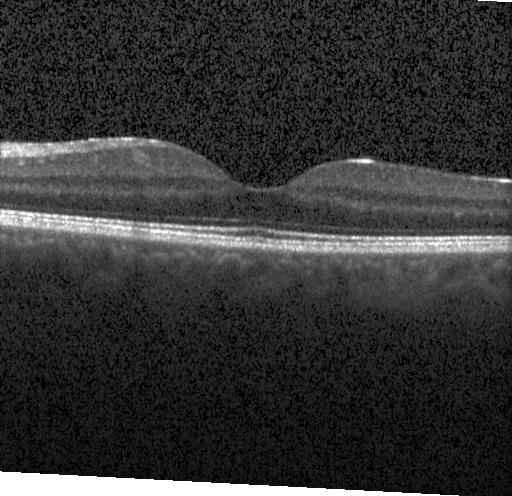

OCT scan showing neither CNV, DME, nor drusen.